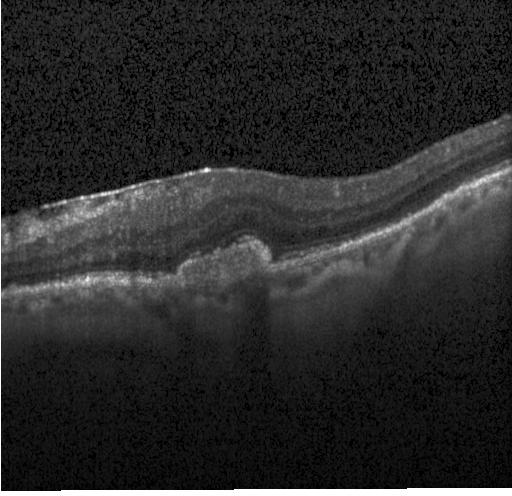

Macular OCT: choroidal neovascularization (CNV).